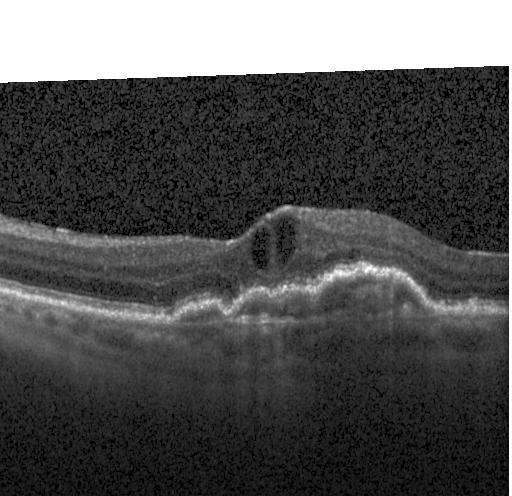

The scan shows a choroidal neovascular membrane.